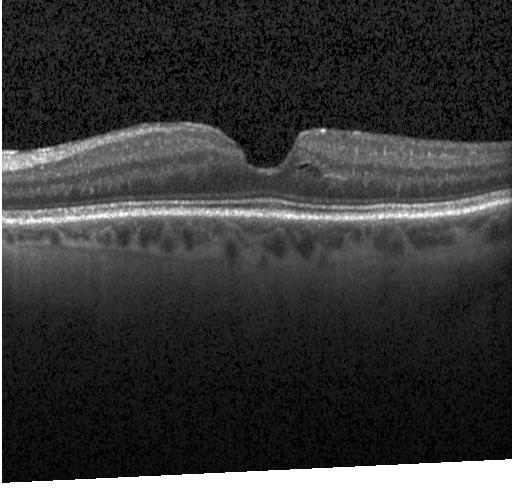

Spectral-domain OCT, retinal OCT cross-section, acquired on a Heidelberg Spectralis.
Impression: diabetic macular edema (DME).